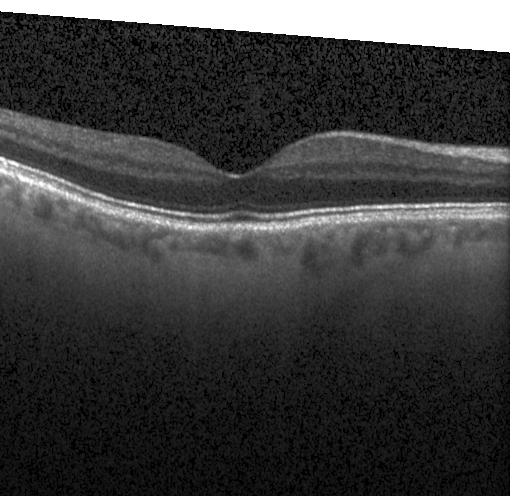

The scan shows no choroidal neovascularization, diabetic macular edema, or drusen.